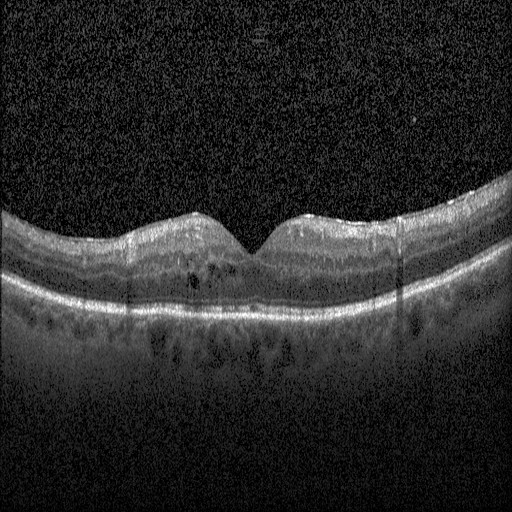
Finding: diabetic macular edema.